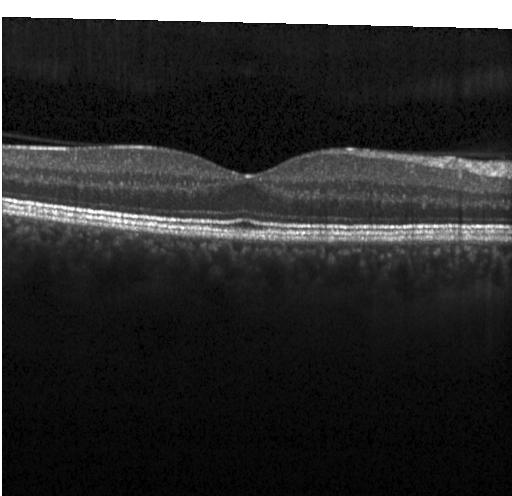 Retinal OCT cross-section — Impression: neither choroidal neovascularization, diabetic macular edema, nor drusen.